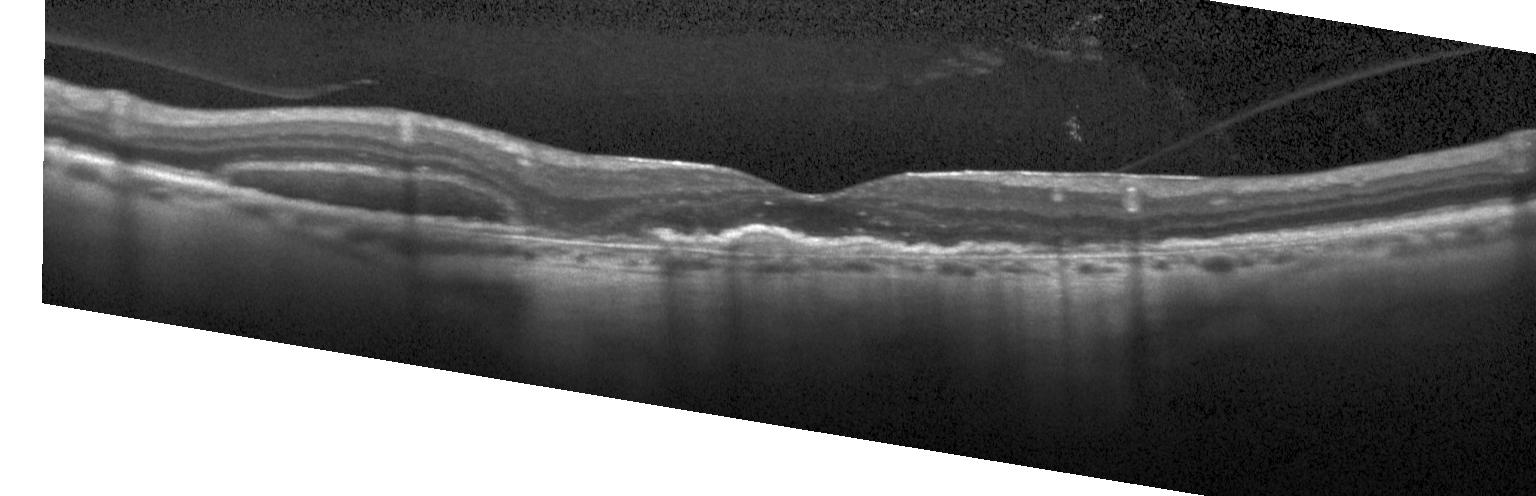

Finding: a choroidal neovascular membrane.